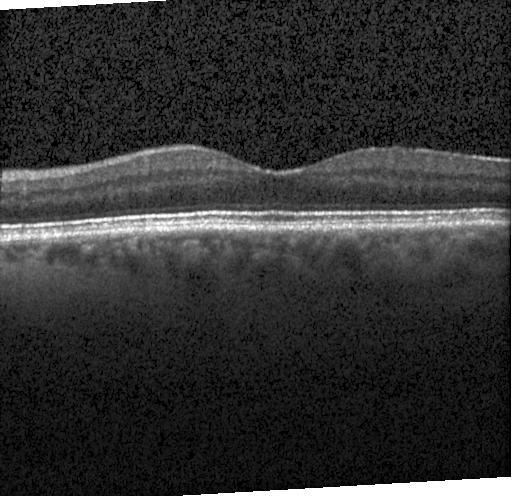 Finding: no evidence of choroidal neovascularization, diabetic macular edema, or drusen.